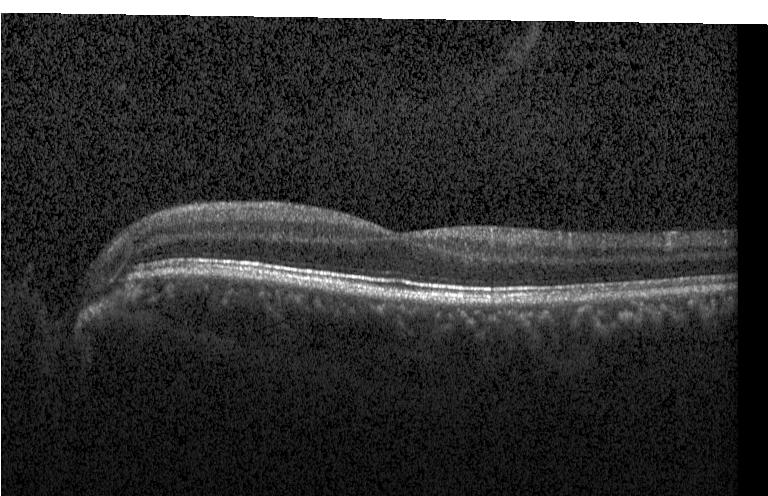
Finding: no evidence of CNV, DME, or drusen.